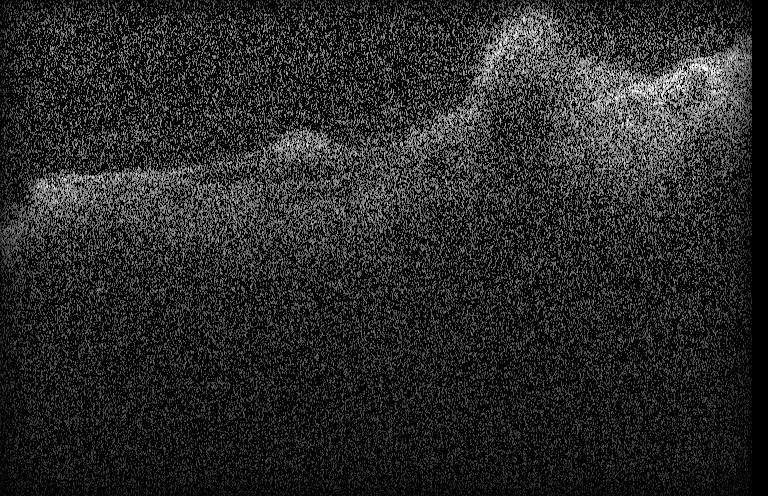
Acquired on a Heidelberg Spectralis, centered on the fovea, optical coherence tomography B-scan — Impression: a choroidal neovascular membrane.